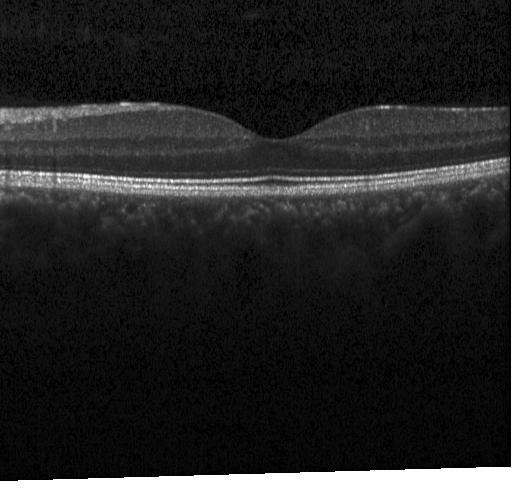

Retinal OCT cross-section — Dx: no evidence of choroidal neovascularization, diabetic macular edema, or drusen.